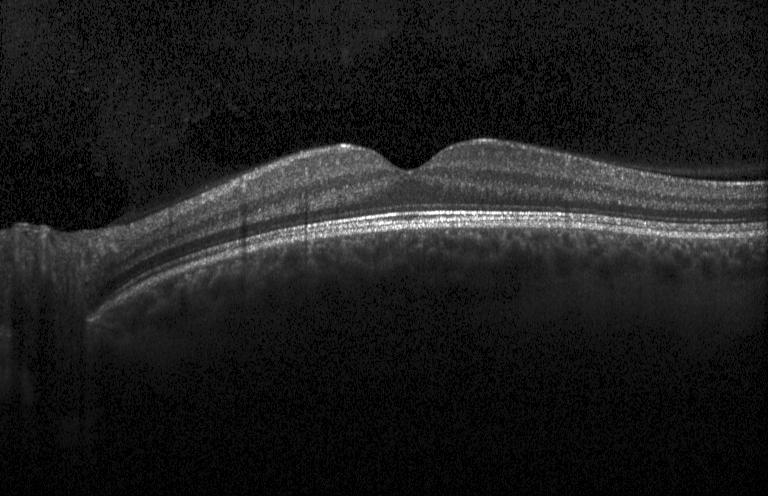
Macular OCT demonstrating no choroidal neovascularization, no diabetic macular edema, and no drusen.